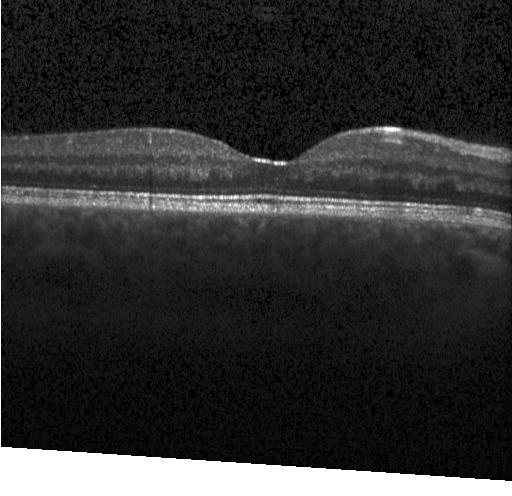
Diagnosis: no CNV, no DME, and no drusen.